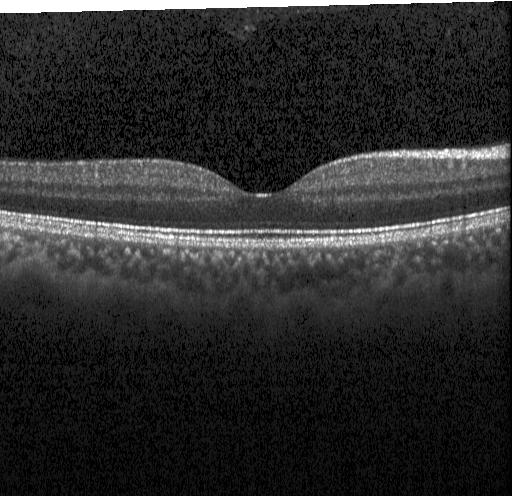 Instrument: Heidelberg Spectralis, spectral-domain optical coherence tomography, centered on the fovea, optical coherence tomography B-scan. Assessment: no choroidal neovascularization, no diabetic macular edema, and no drusen.